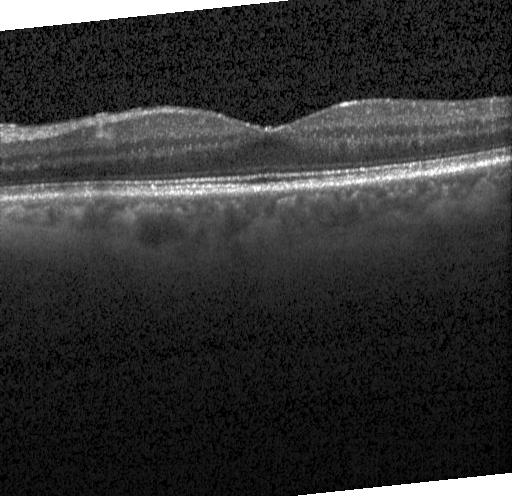
Heidelberg Spectralis OCT system; retinal OCT B-scan
Diagnosis: no choroidal neovascularization, diabetic macular edema, or drusen.